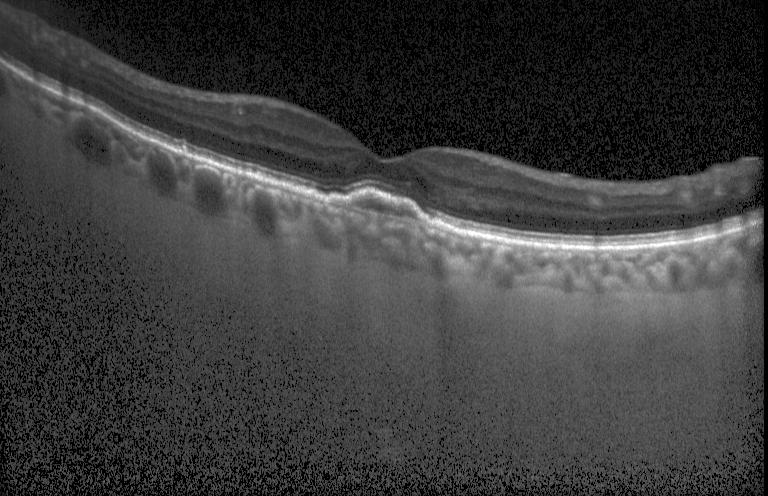 Spectral-domain OCT B-scan: a choroidal neovascular membrane.